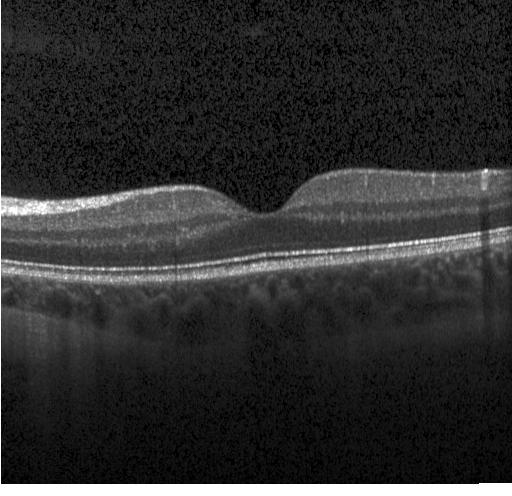

OCT B-scan — Diagnosis: no CNV, DME, or drusen.